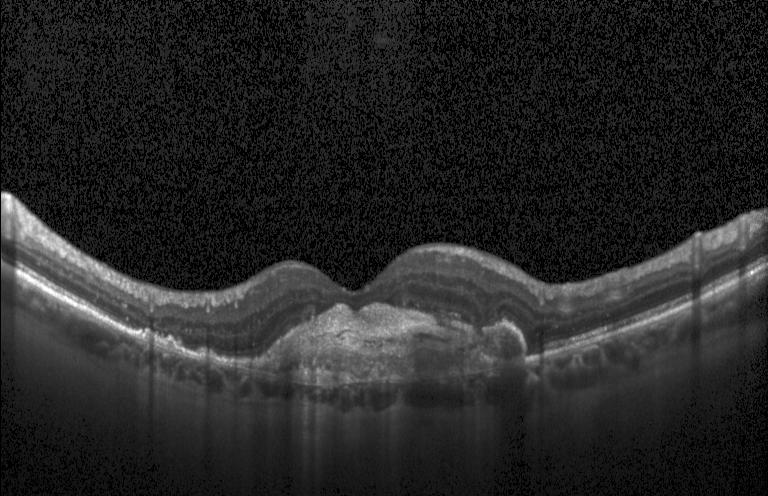

This B-scan demonstrates a choroidal neovascular membrane.